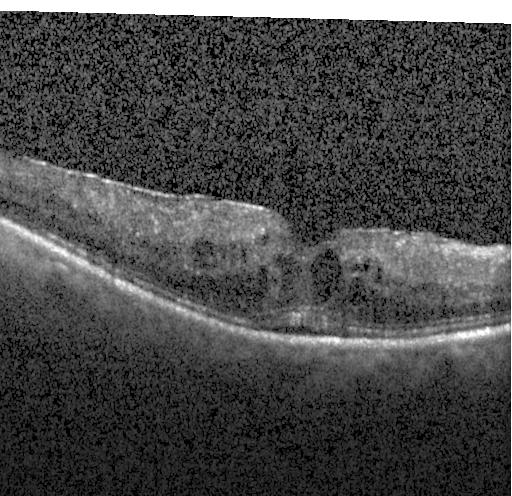
Retinal OCT B-scan · SD-OCT · centered on the fovea. This B-scan demonstrates DME.